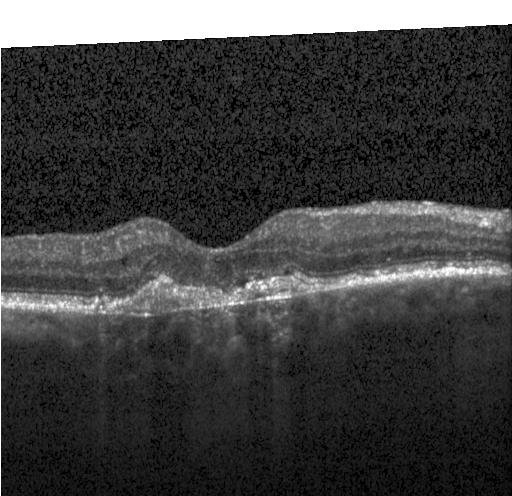 OCT finding: a choroidal neovascular membrane.